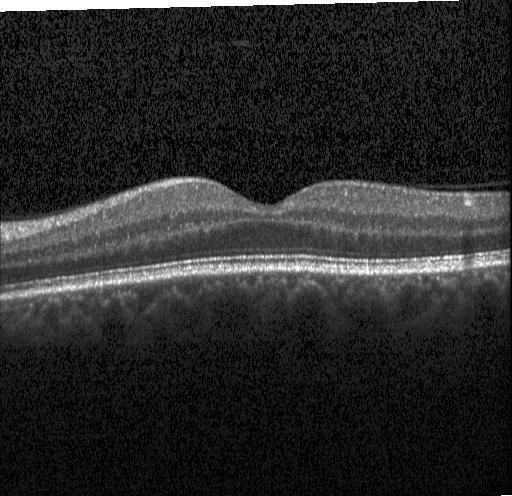 SD-OCT · horizontal scan through the fovea · optical coherence tomography scan · Heidelberg Spectralis OCT system
Impression: no choroidal neovascularization, no diabetic macular edema, and no drusen.